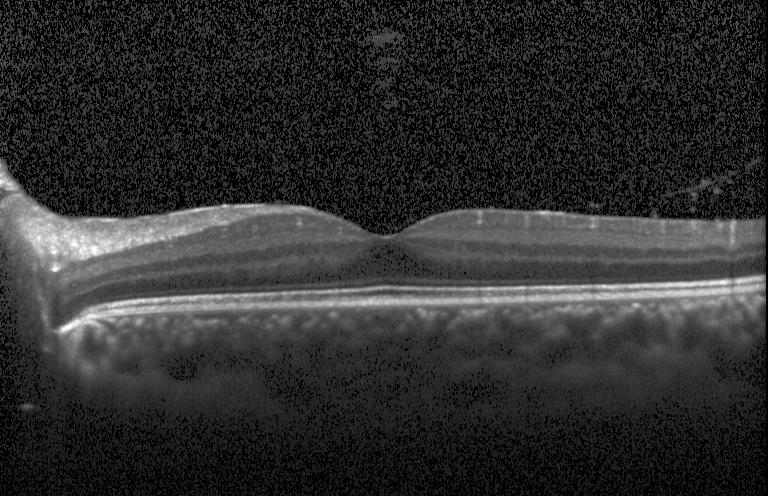

Finding: no evidence of choroidal neovascularization, diabetic macular edema, or drusen.